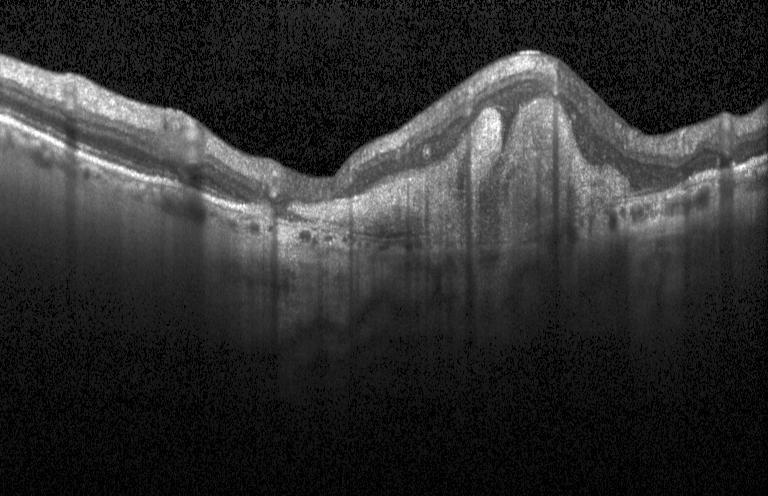
Impression: a choroidal neovascular membrane.